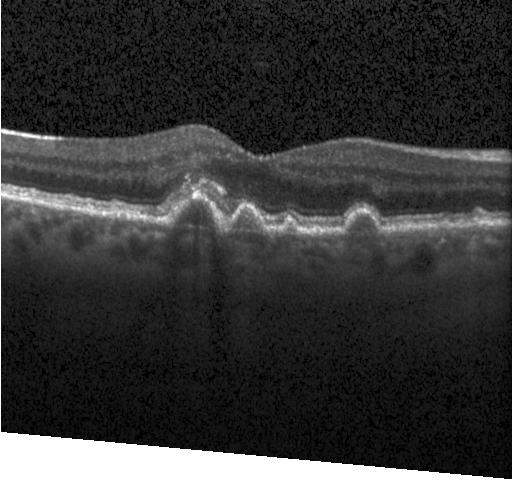 Macular OCT: drusen.